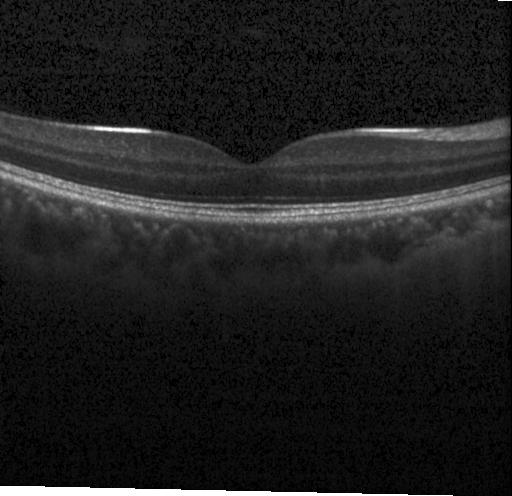
Spectral-domain OCT; horizontal scan through the fovea; acquired on a Heidelberg Spectralis; optical coherence tomography scan — Impression: no choroidal neovascularization, no diabetic macular edema, and no drusen.